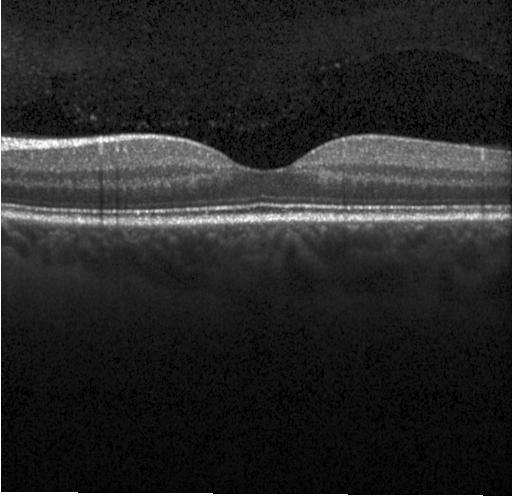
OCT B-scan — Diagnosis: no choroidal neovascularization, diabetic macular edema, or drusen.